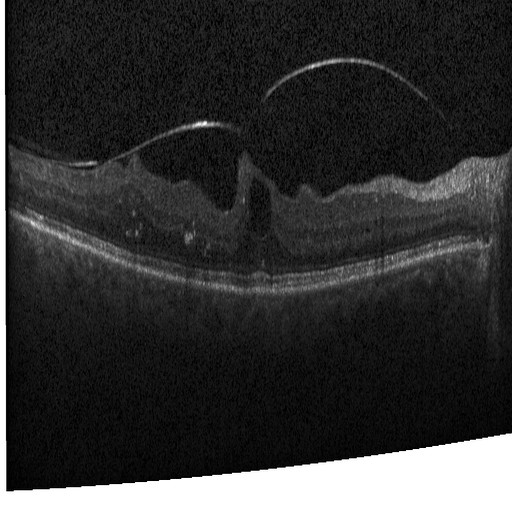 This B-scan demonstrates diabetic macular edema (DME).